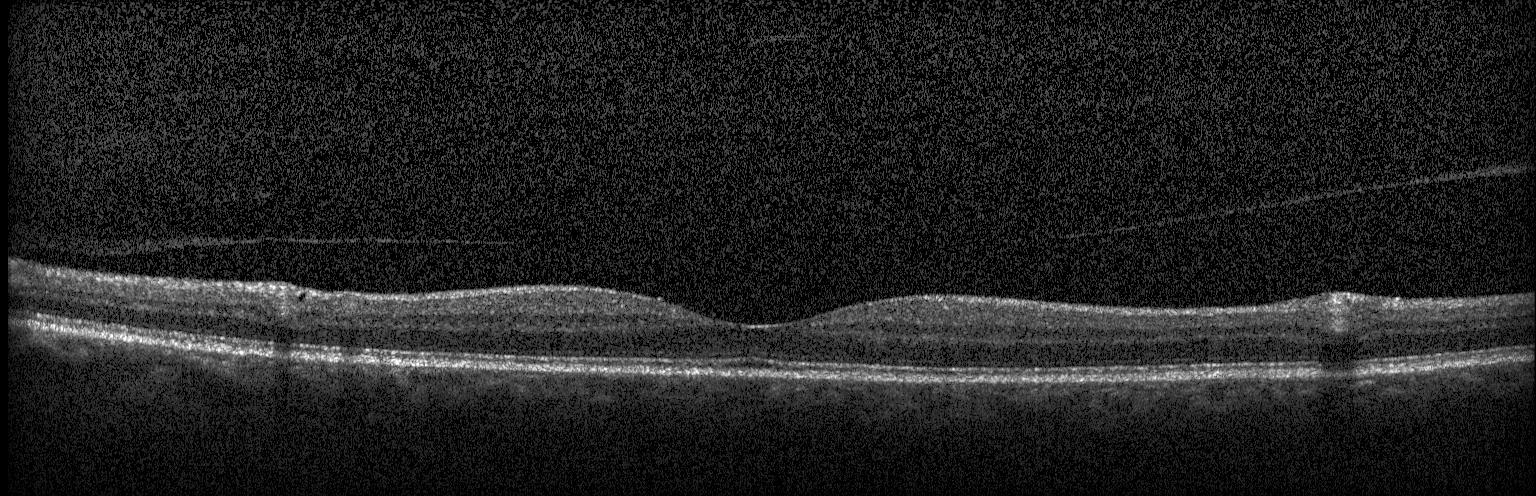

No evidence of CNV, DME, or drusen.